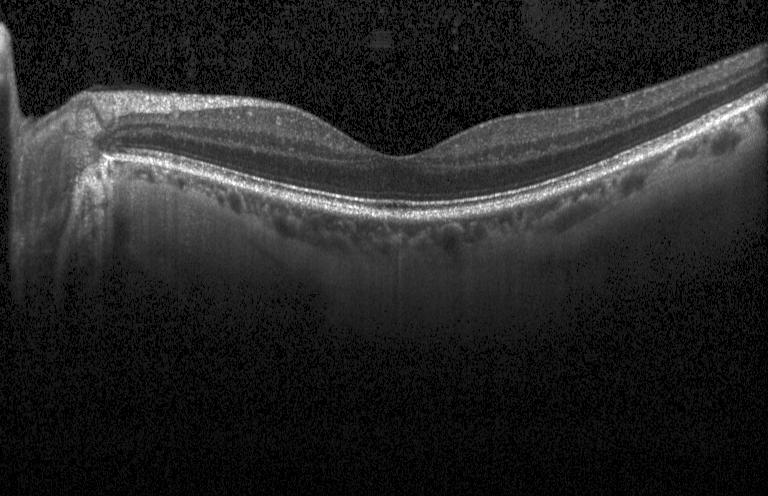

Heidelberg Spectralis. Spectral-domain optical coherence tomography. Optical coherence tomography B-scan.
Macular OCT: neither choroidal neovascularization, diabetic macular edema, nor drusen.